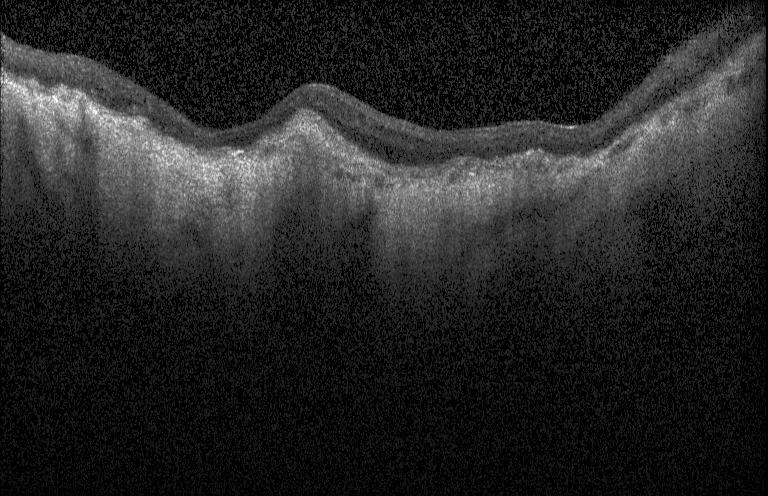
OCT B-scan showing choroidal neovascularization.